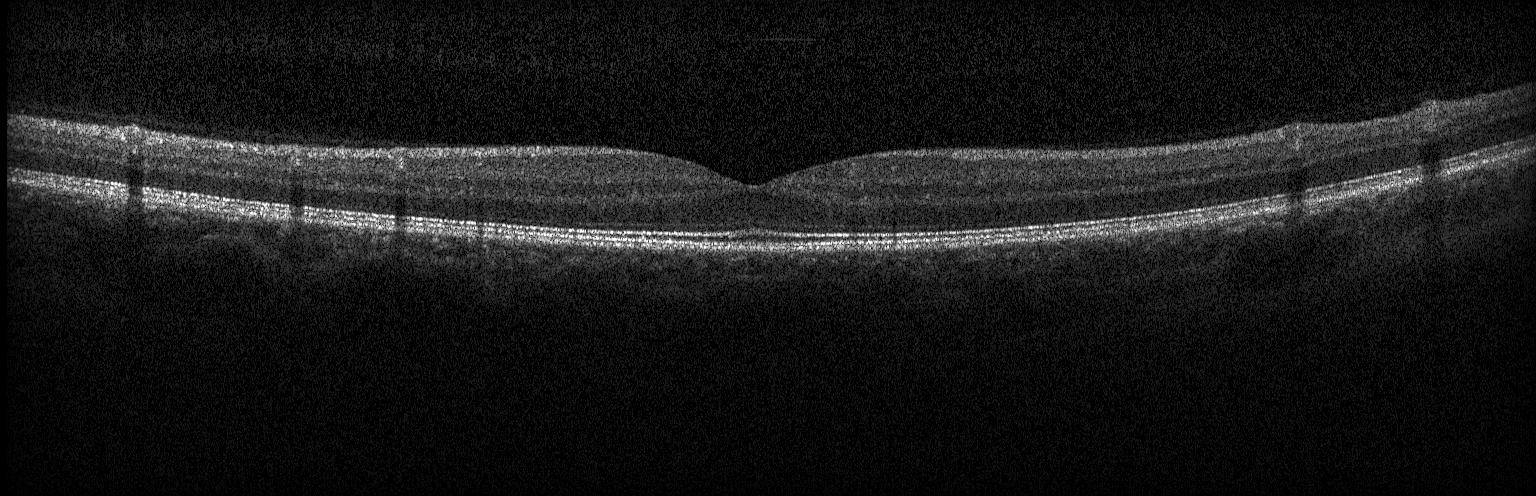 Optical coherence tomography B-scan. Spectral-domain OCT.
Finding: no evidence of choroidal neovascularization, diabetic macular edema, or drusen.